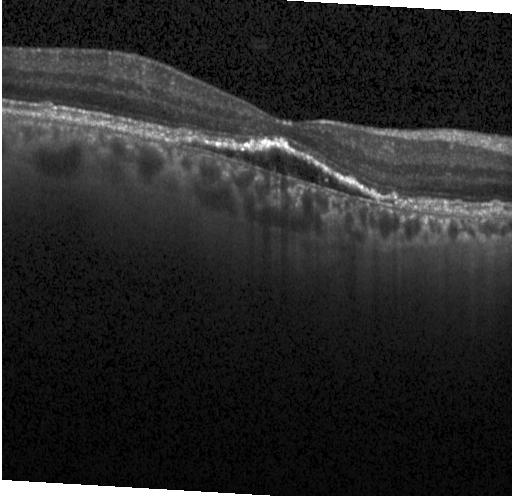
Spectral-domain OCT, acquired on a Heidelberg Spectralis, retinal OCT cross-section. Dx: a choroidal neovascular membrane.